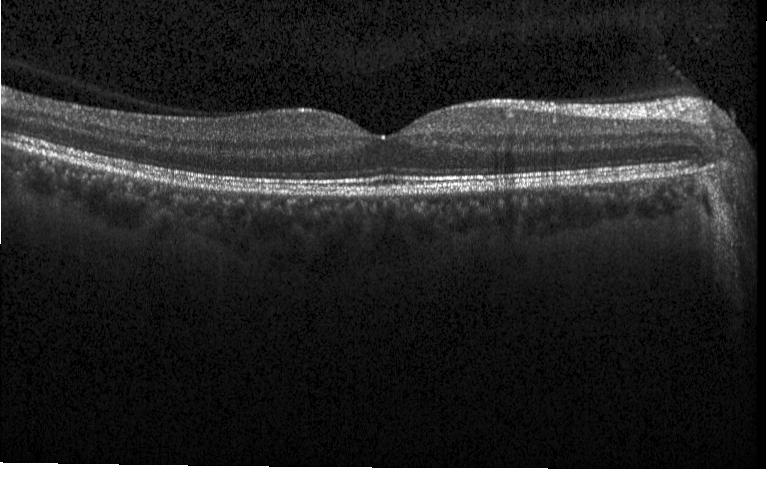 SD-OCT · fovea-centered · retinal OCT B-scan — Macular OCT: no choroidal neovascularization, no diabetic macular edema, and no drusen.